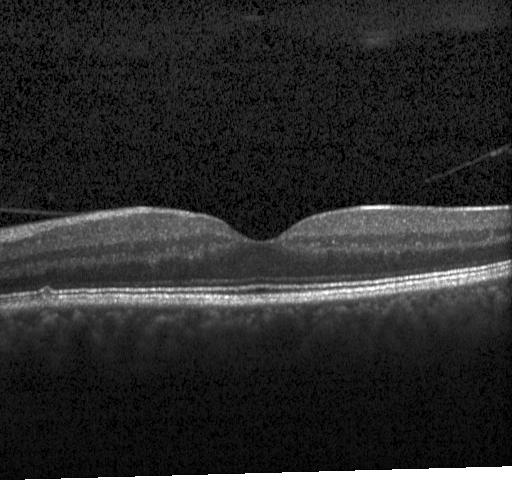
Macular OCT: no CNV, DME, or drusen.